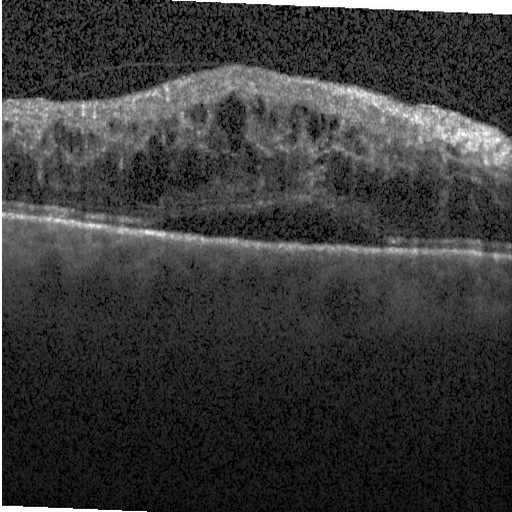

Through the macula; OCT B-scan; spectral-domain OCT — Dx: diabetic macular edema.